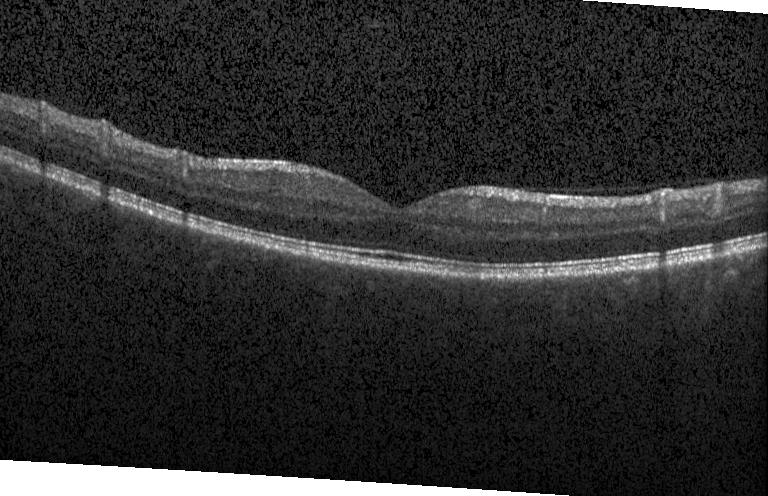 Retinal OCT B-scan.
The scan shows no CNV, no DME, and no drusen.